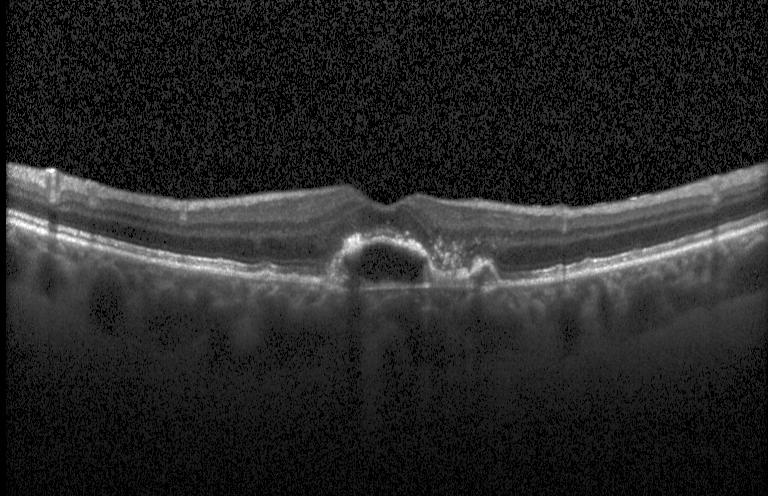

OCT B-scan; Heidelberg Spectralis OCT system; SD-OCT — Impression: choroidal neovascularization (CNV).